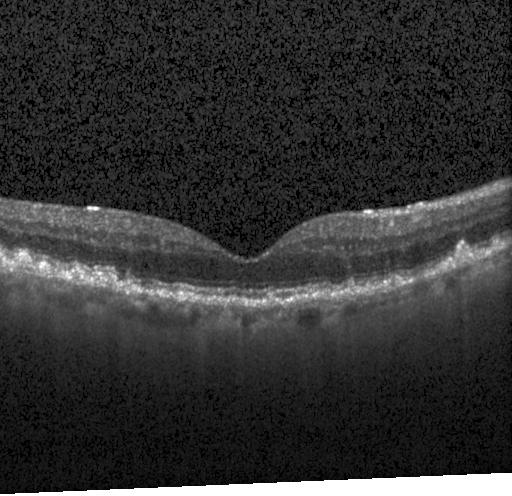

Optical coherence tomography scan; centered on the fovea — The scan shows sub-RPE drusenoid deposits.